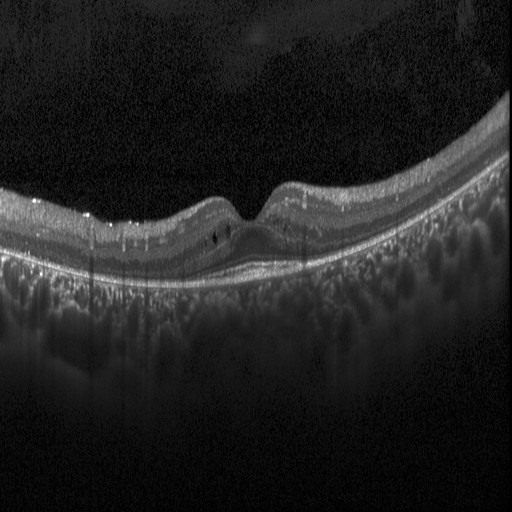 Acquired on a Heidelberg Spectralis, spectral-domain OCT, retinal OCT cross-section.
Finding: diabetic macular edema (DME).